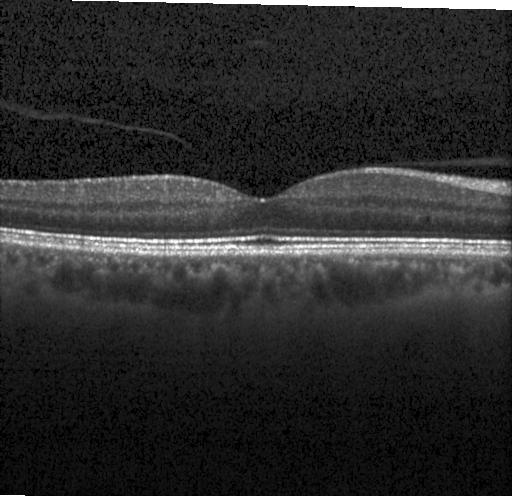

Heidelberg Spectralis, spectral-domain optical coherence tomography, optical coherence tomography B-scan — Diagnosis: no CNV, DME, or drusen.